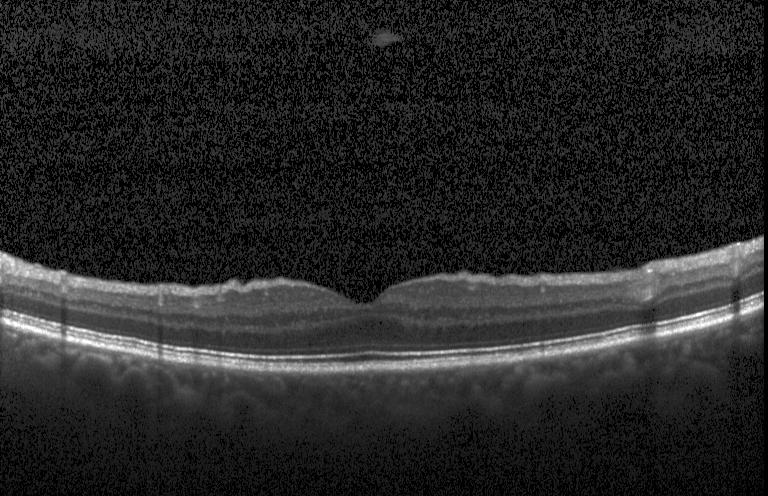
Spectral-domain optical coherence tomography; retinal OCT B-scan; horizontal scan through the fovea; acquired on a Heidelberg Spectralis.
Diagnosis: neither choroidal neovascularization, diabetic macular edema, nor drusen.